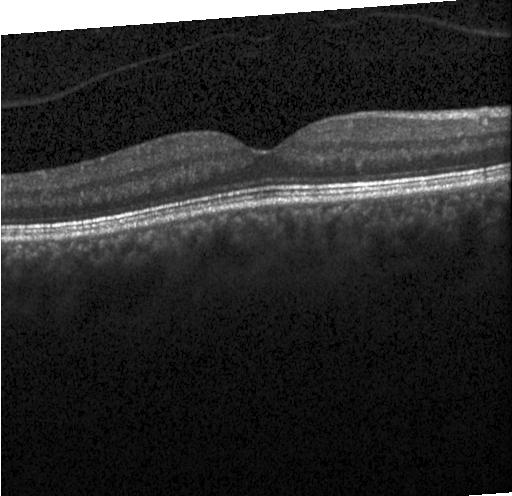
Spectral-domain optical coherence tomography, OCT B-scan, acquired on a Heidelberg Spectralis
Impression: no CNV, no DME, and no drusen.